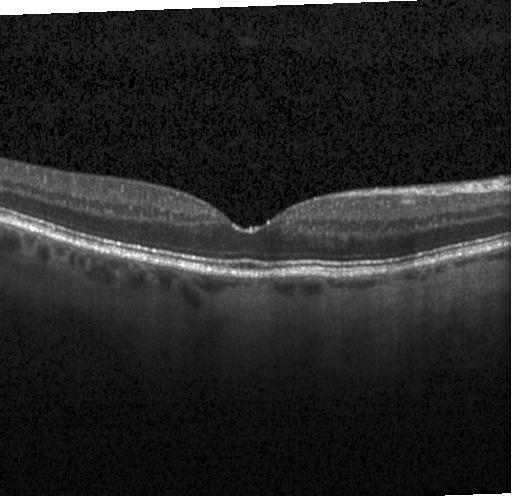
Retinal OCT B-scan.
Macular OCT: no evidence of choroidal neovascularization, diabetic macular edema, or drusen.